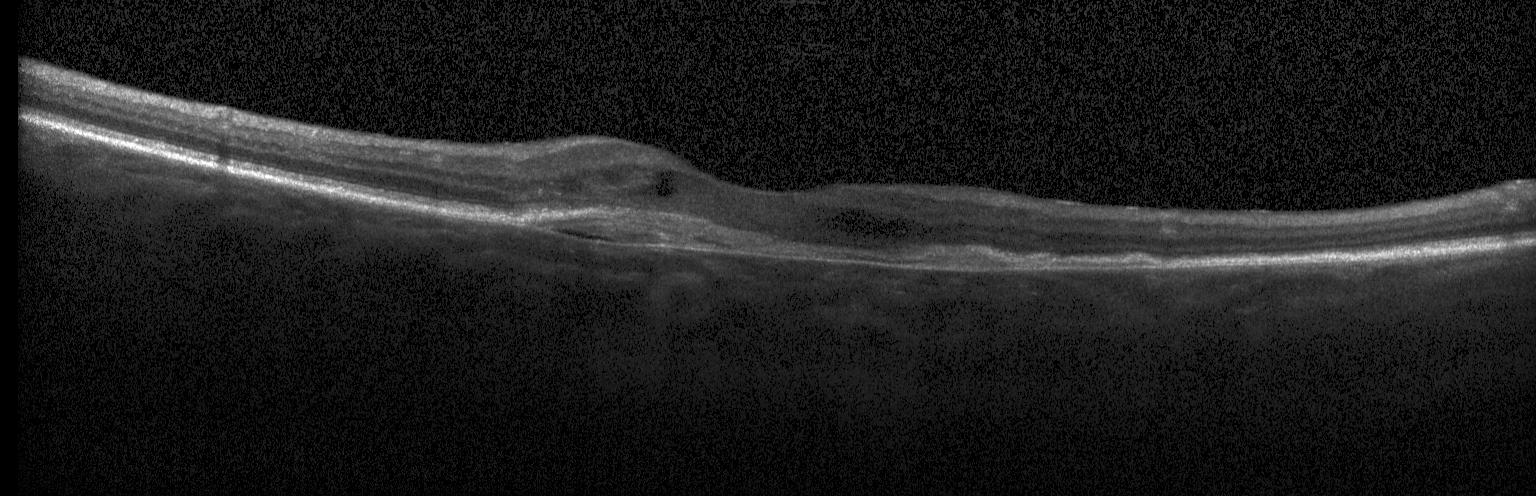

Spectral-domain optical coherence tomography · optical coherence tomography scan · Heidelberg Spectralis
Assessment: choroidal neovascularization (CNV).